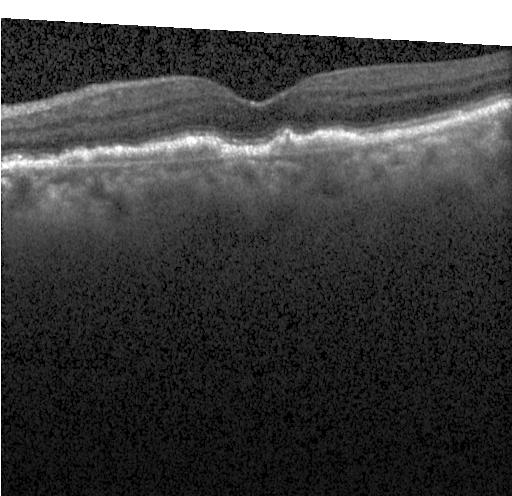 Choroidal neovascularization (CNV).